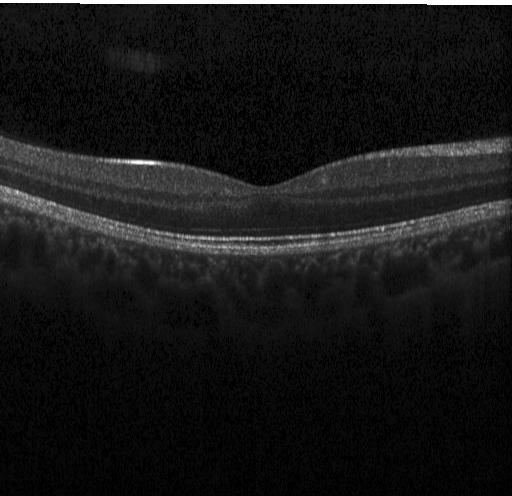

Impression: neither CNV, DME, nor drusen.